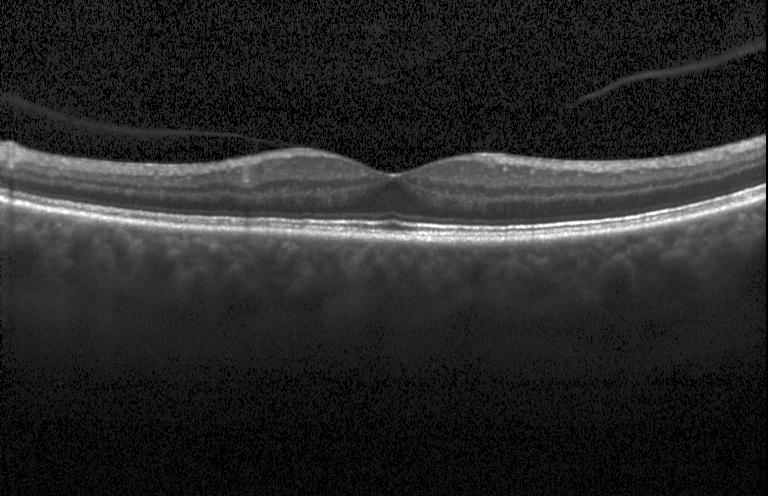

No evidence of choroidal neovascularization, diabetic macular edema, or drusen.